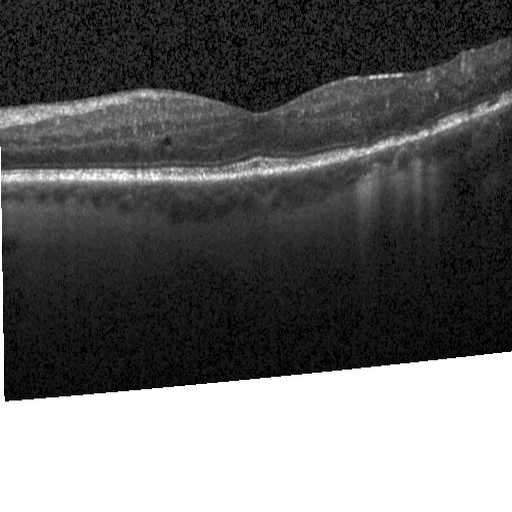 SD-OCT, instrument: Heidelberg Spectralis, optical coherence tomography scan, centered on the fovea — Diagnosis: diabetic macular edema.